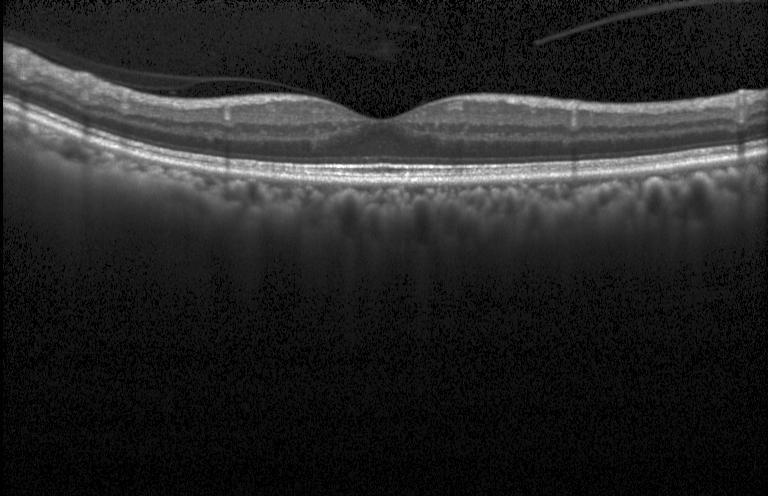

OCT line scan, horizontal scan through the fovea, SD-OCT
Finding: neither choroidal neovascularization, diabetic macular edema, nor drusen.